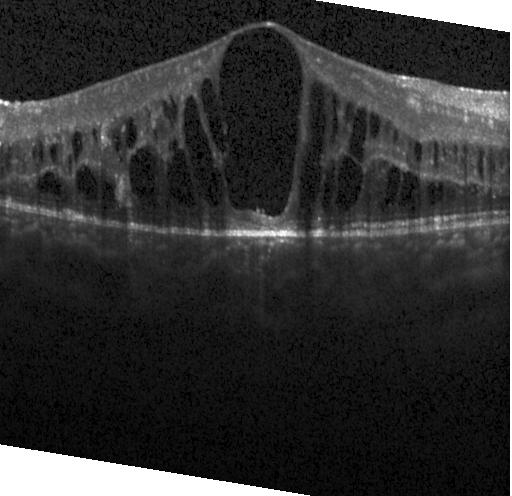 OCT B-scan. Assessment: diabetic macular edema (DME).